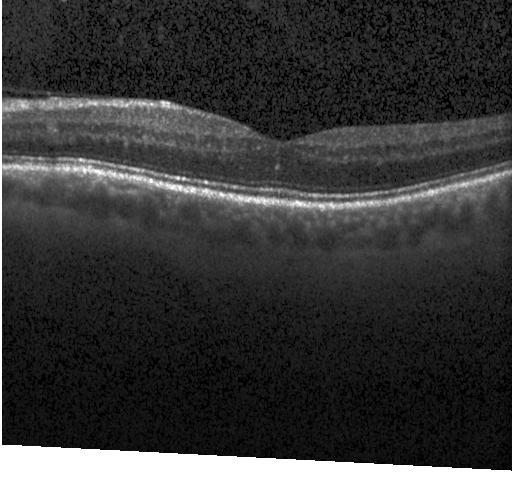
Macular OCT demonstrating no evidence of choroidal neovascularization, diabetic macular edema, or drusen.